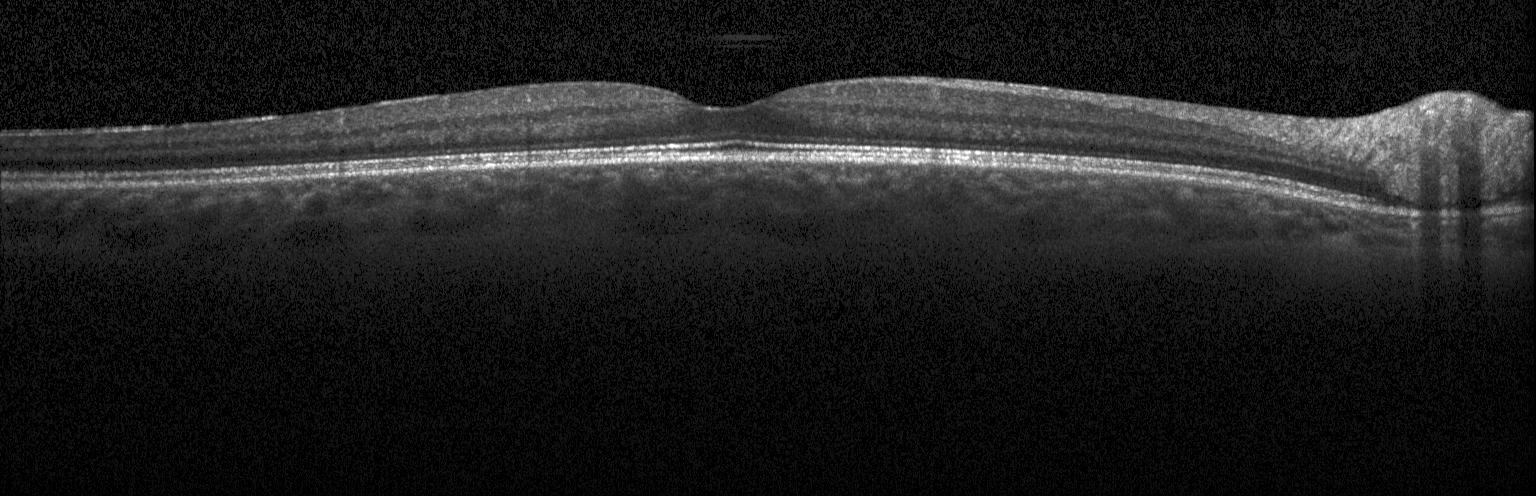
Impression: no choroidal neovascularization, no diabetic macular edema, and no drusen.